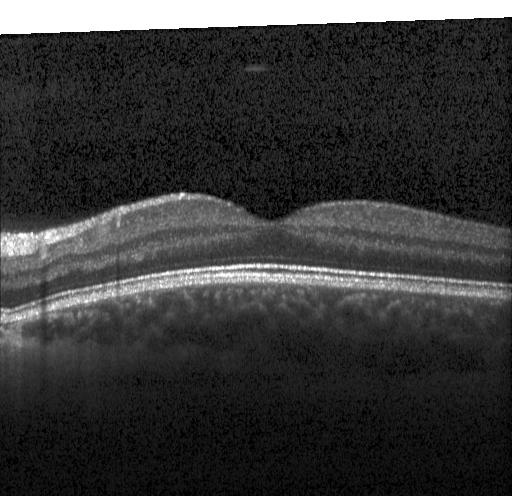

Macular scan; Heidelberg Spectralis OCT system; spectral-domain OCT; retinal OCT B-scan
Finding: no CNV, no DME, and no drusen.